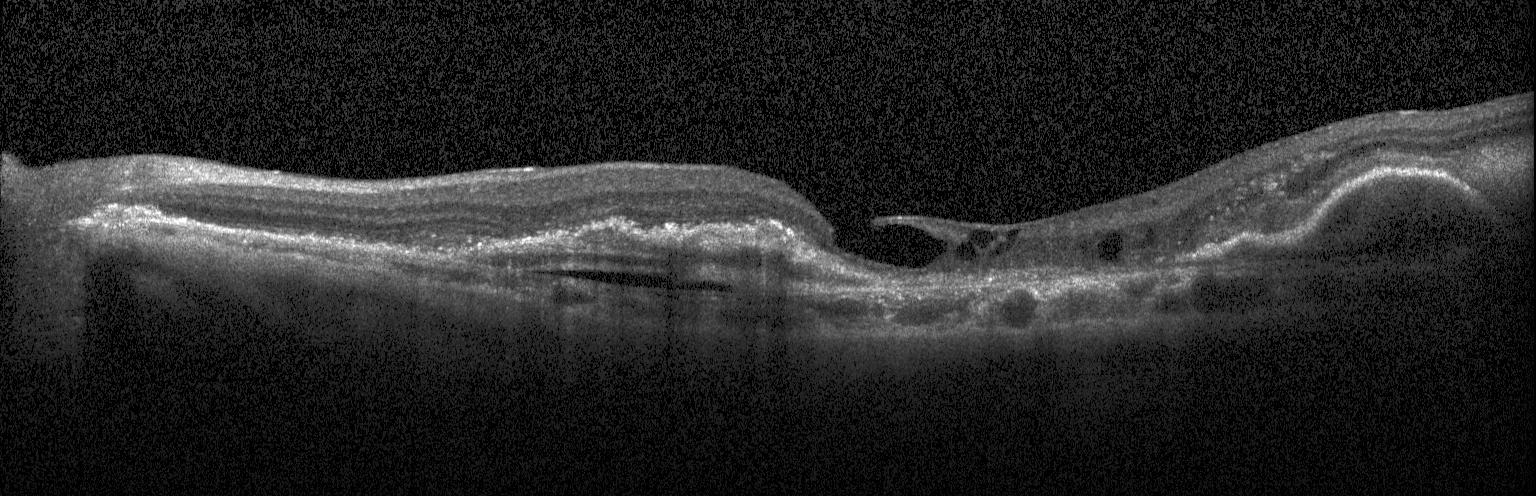

Retinal OCT B-scan
Finding: choroidal neovascularization.